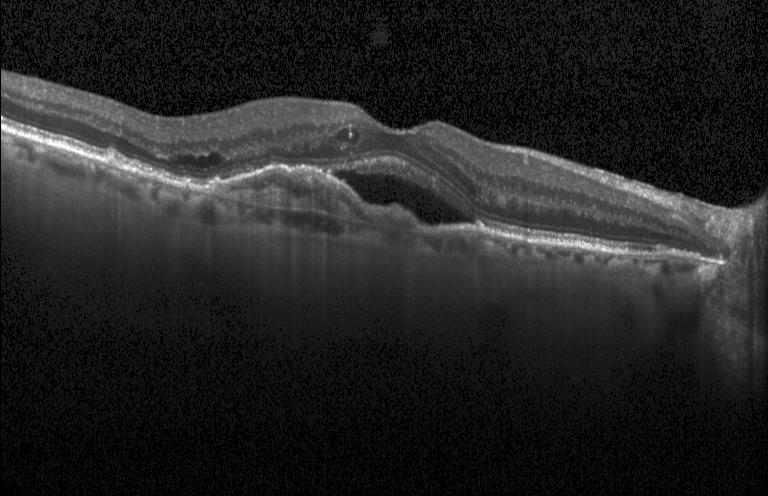
Spectral-domain optical coherence tomography. Optical coherence tomography scan. Through the macula
The scan shows choroidal neovascularization.